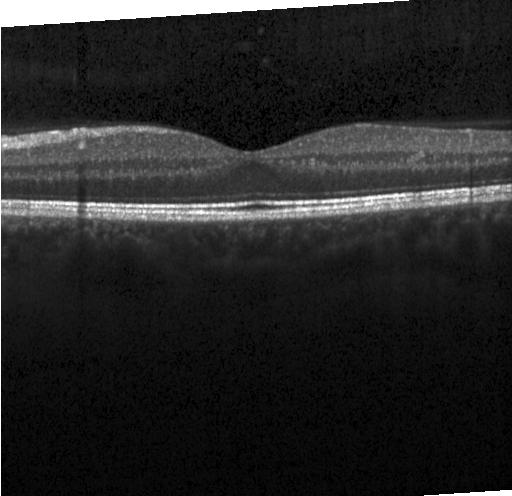 Heidelberg Spectralis, OCT line scan, through the macula
This B-scan demonstrates neither choroidal neovascularization, diabetic macular edema, nor drusen.